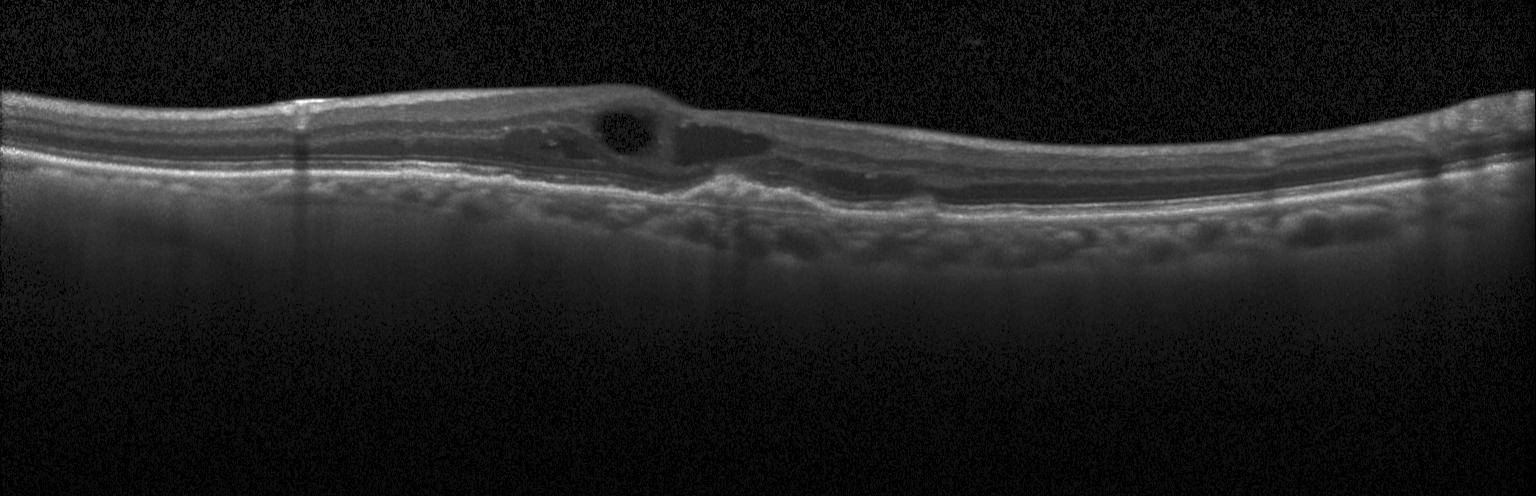
Diagnosis: a choroidal neovascular membrane.